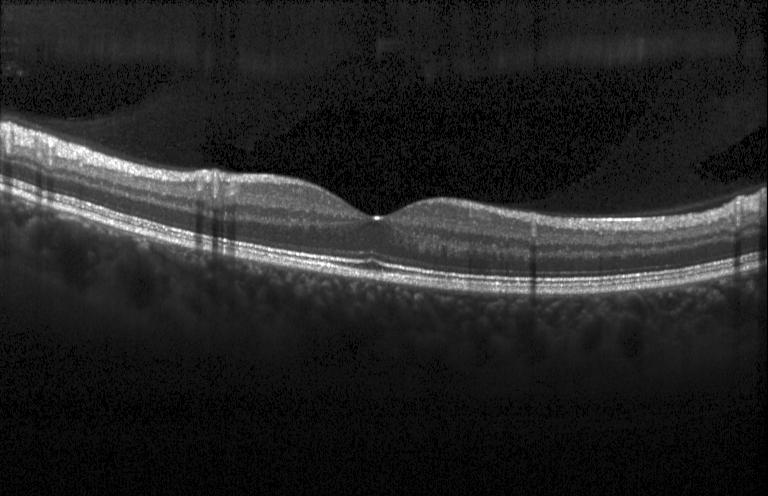

Optical coherence tomography scan; spectral-domain OCT.
This B-scan demonstrates neither choroidal neovascularization, diabetic macular edema, nor drusen.